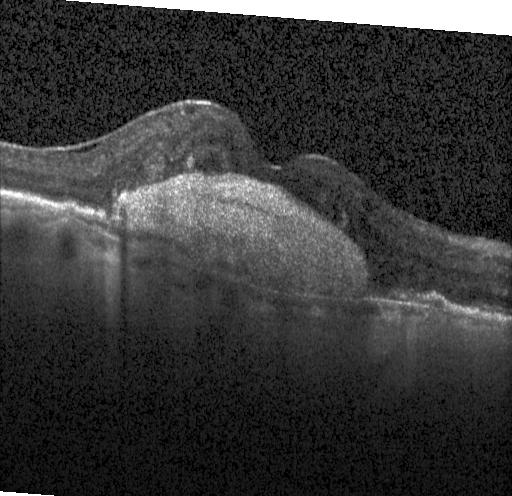 Spectral-domain OCT; instrument: Heidelberg Spectralis; OCT line scan — Finding: CNV.